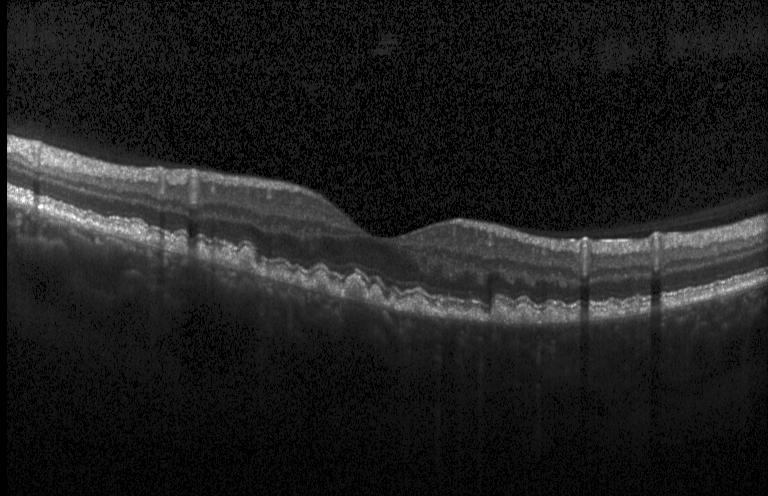
Centered on the fovea; OCT line scan; instrument: Heidelberg Spectralis.
Diagnosis: multiple drusen.